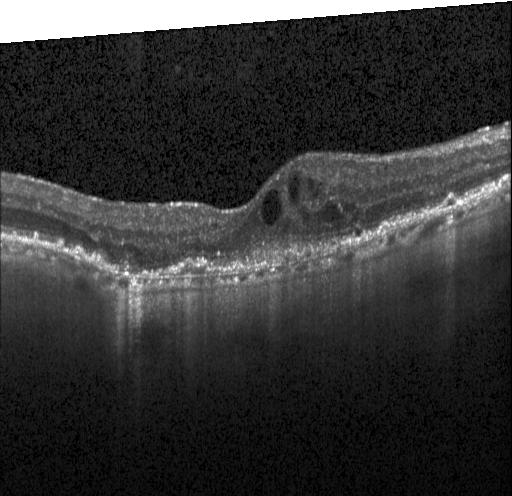
Impression: choroidal neovascularization.